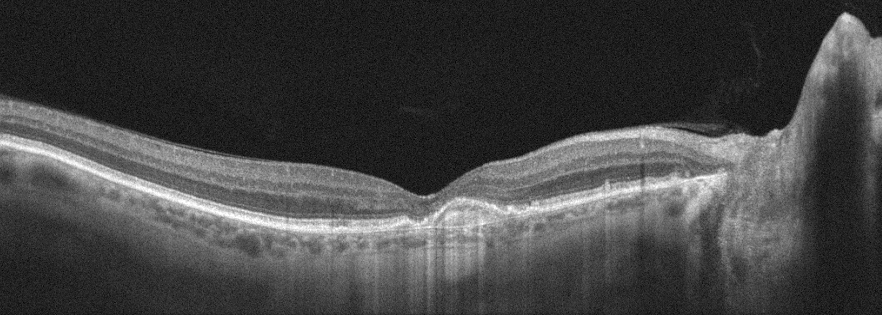
Retinal OCT B-scan · right eye
Dx: age-related macular degeneration (AMD).